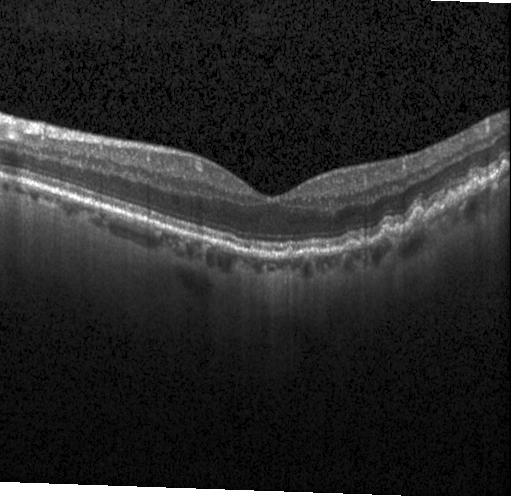
Instrument: Heidelberg Spectralis, OCT line scan — Diagnosis: sub-RPE drusenoid deposits.